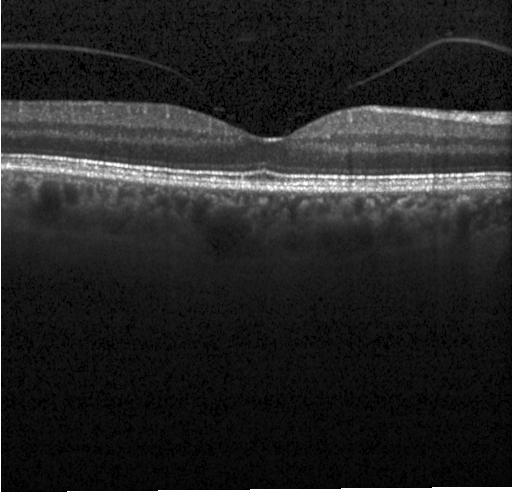 Assessment: no evidence of choroidal neovascularization, diabetic macular edema, or drusen.